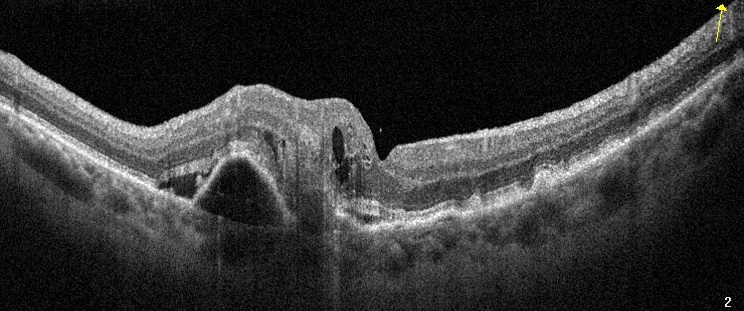

Retinal OCT cross-section — Diagnosis: age-related macular degeneration (AMD).